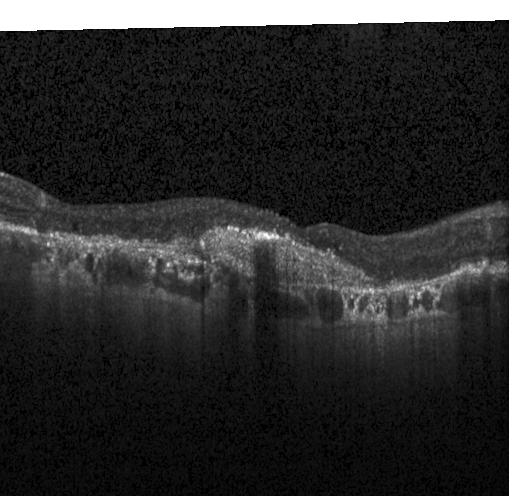 OCT B-scan. Diagnosis: choroidal neovascularization (CNV).